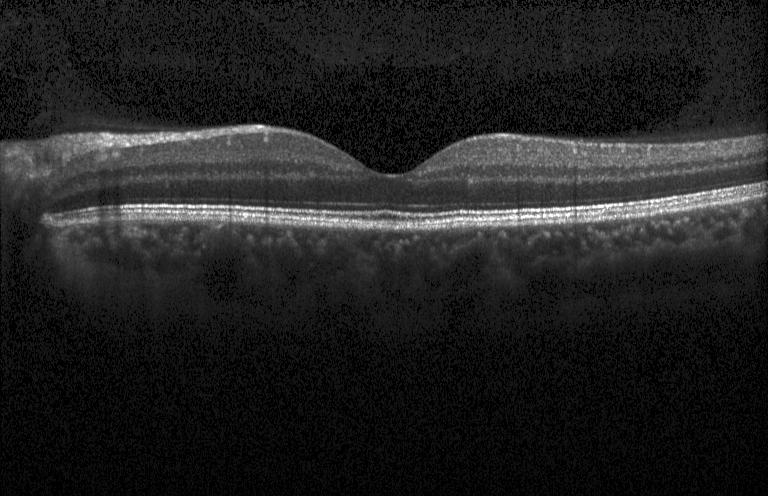 Retinal OCT cross-section — The scan shows neither CNV, DME, nor drusen.